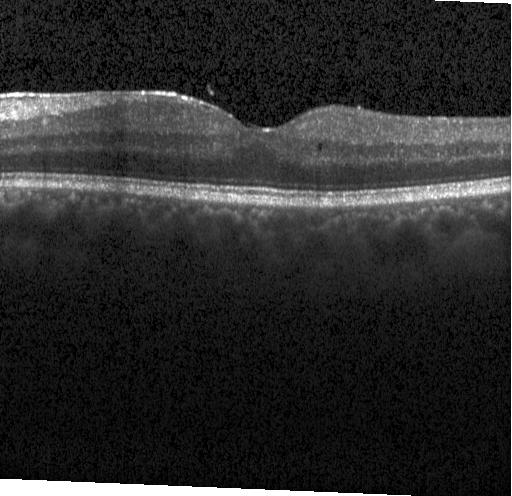 Through the macula. Optical coherence tomography B-scan. Diabetic macular edema (DME).